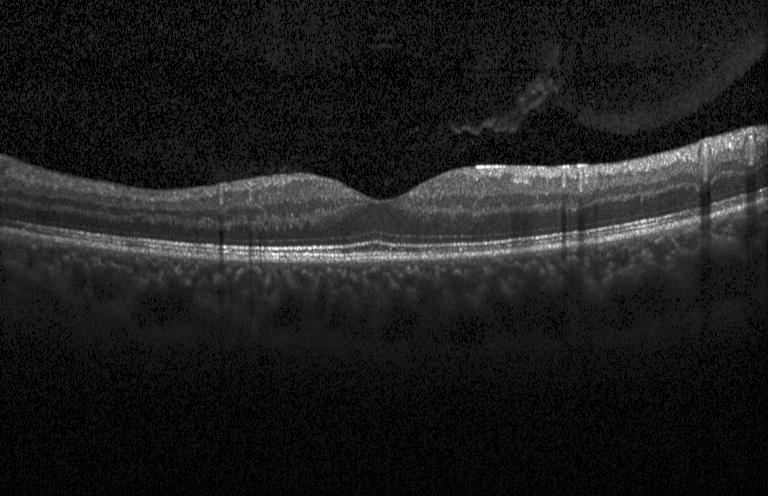
OCT finding: neither choroidal neovascularization, diabetic macular edema, nor drusen.